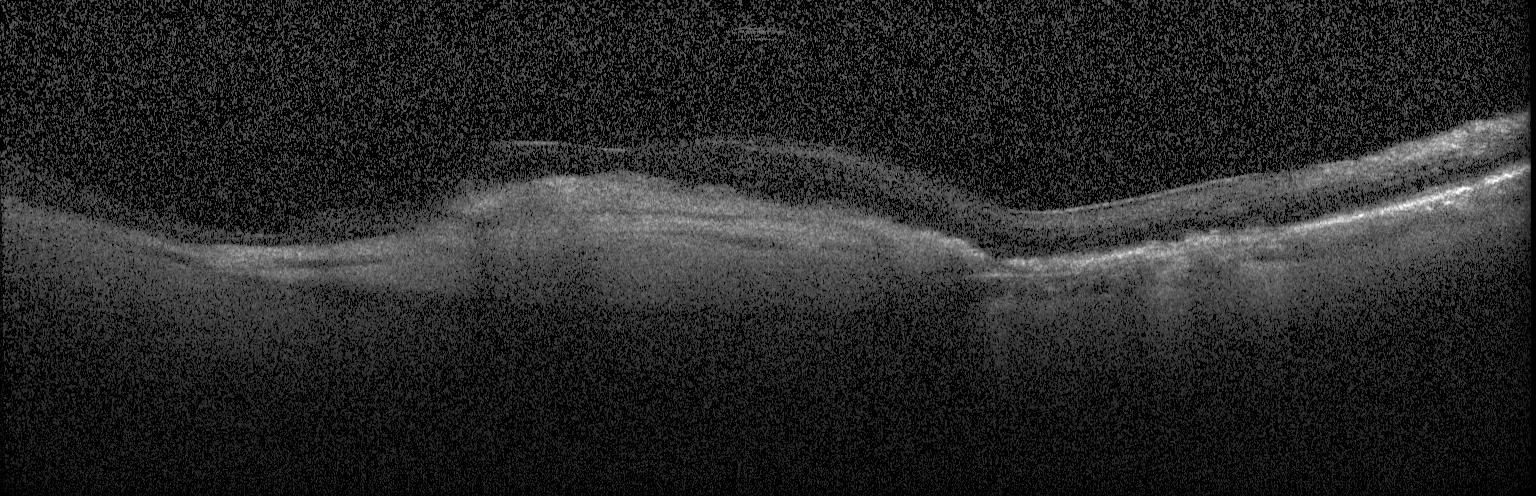
Centered on the fovea. OCT B-scan. Diagnosis: a choroidal neovascular membrane.